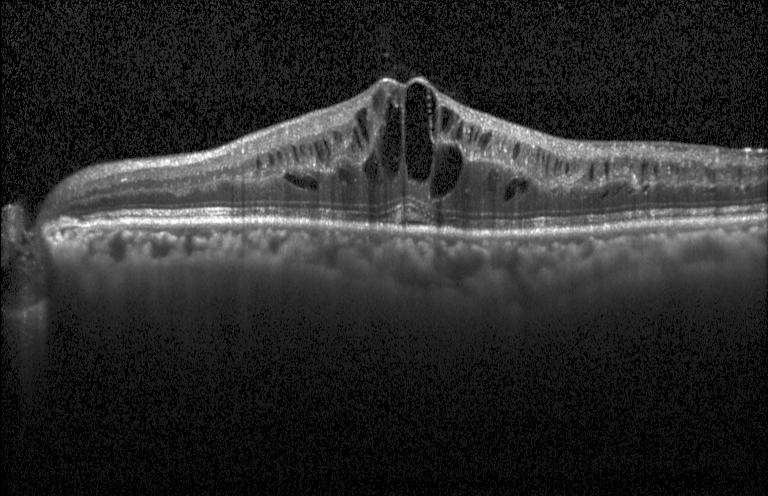 OCT B-scan
The scan shows diabetic macular edema (DME).